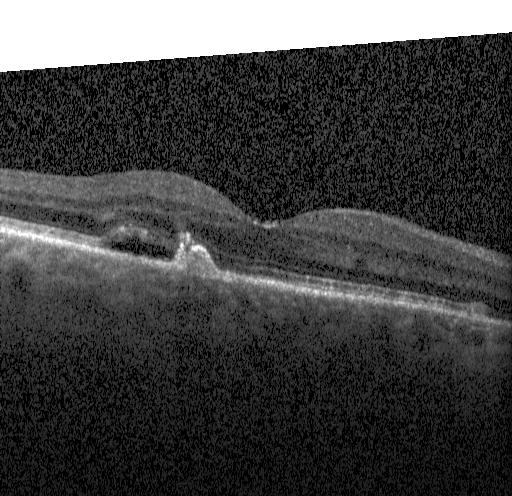

Spectral-domain OCT. OCT line scan. Dx: a choroidal neovascular membrane.